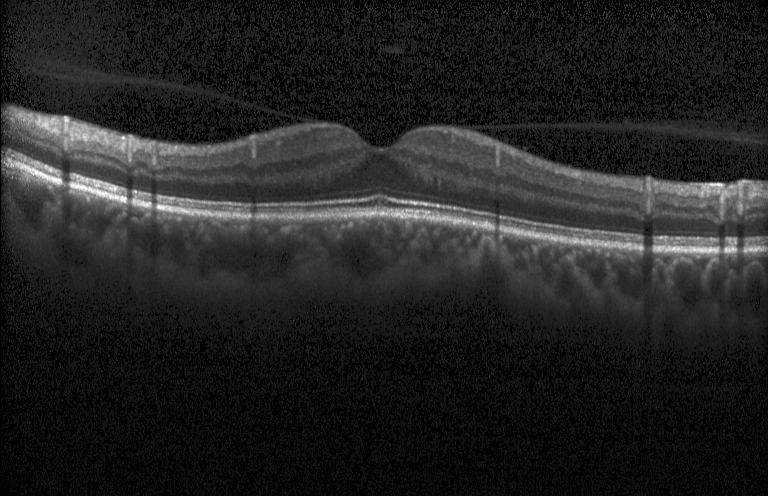
OCT B-scan, horizontal scan through the fovea, spectral-domain OCT, Heidelberg Spectralis. Impression: neither choroidal neovascularization, diabetic macular edema, nor drusen.